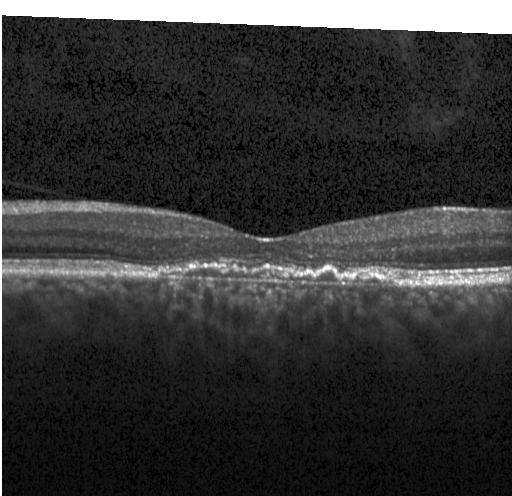 Assessment: CNV.